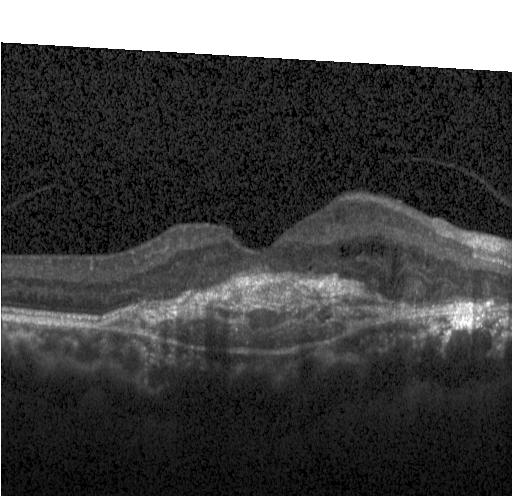

Retinal OCT B-scan — Diagnosis: a choroidal neovascular membrane.